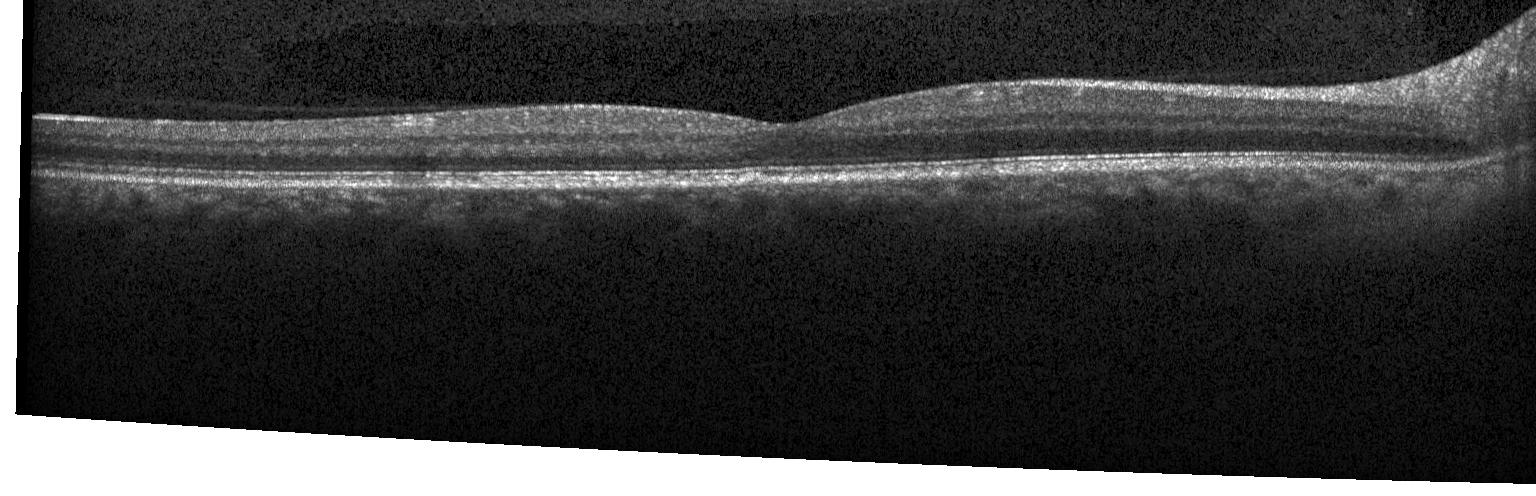

OCT B-scan, through the macula, SD-OCT.
Impression: no evidence of choroidal neovascularization, diabetic macular edema, or drusen.